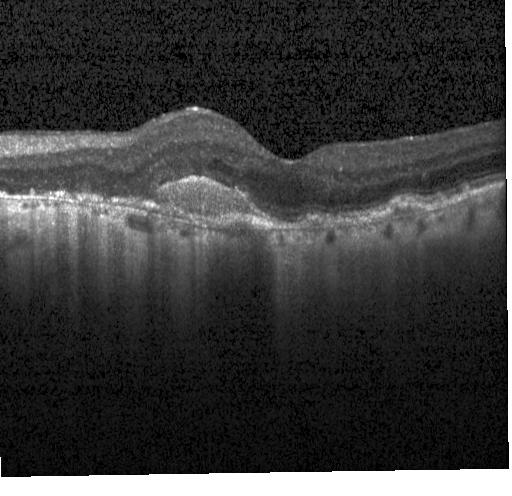 Retinal OCT cross-section
OCT finding: choroidal neovascularization.